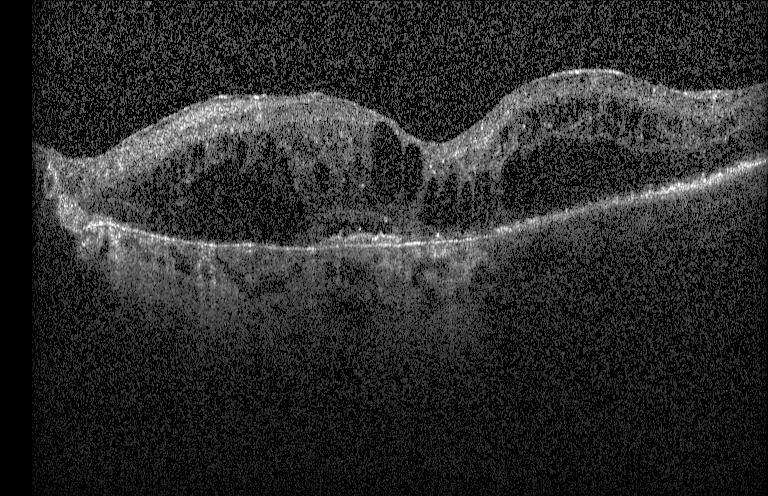 Retinal OCT B-scan.
Dx: a choroidal neovascular membrane.